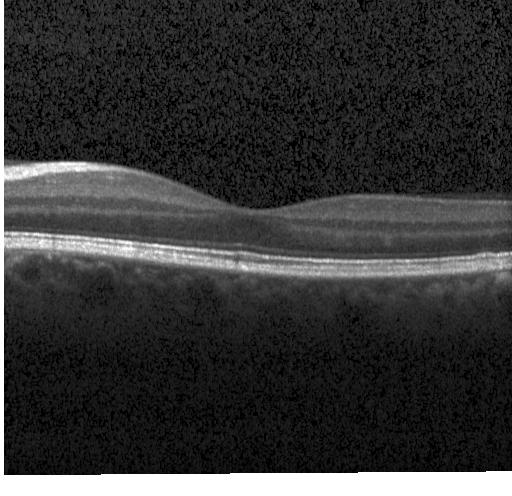
Instrument: Heidelberg Spectralis, through the macula, spectral-domain OCT, retinal OCT B-scan. Finding: neither choroidal neovascularization, diabetic macular edema, nor drusen.